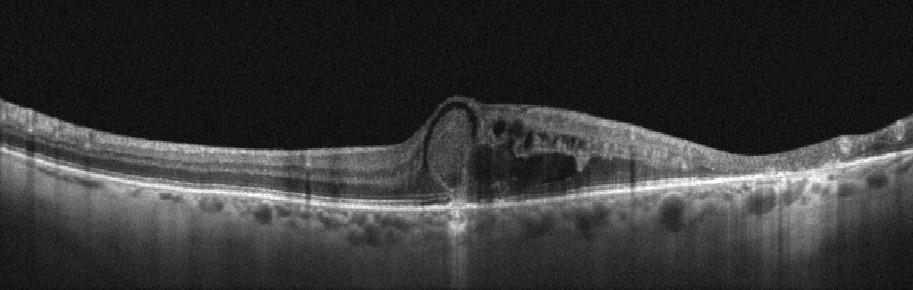 Fovea-centered. Retinal OCT B-scan. Optovue Avanti RTVue XR — Diagnosis: retinal vein occlusion.